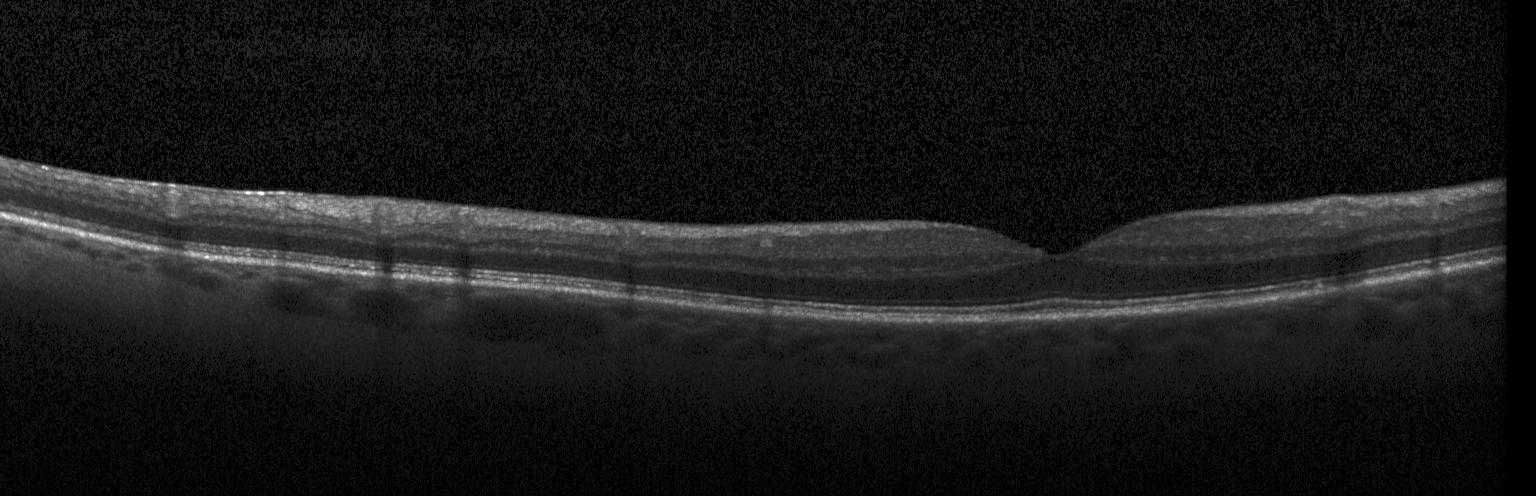

Dx: no evidence of choroidal neovascularization, diabetic macular edema, or drusen.